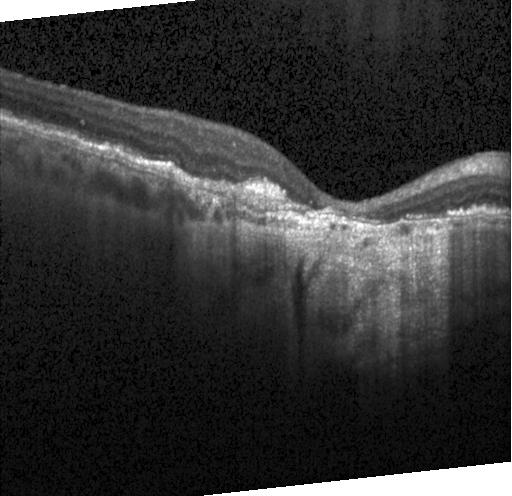 Spectral-domain OCT; Heidelberg Spectralis; horizontal scan through the fovea; optical coherence tomography B-scan.
OCT finding: CNV.